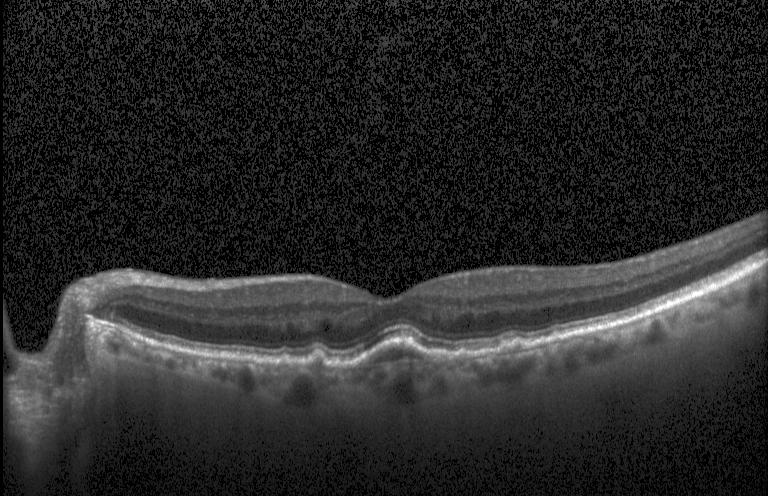 Optical coherence tomography scan.
Finding: choroidal neovascularization (CNV).